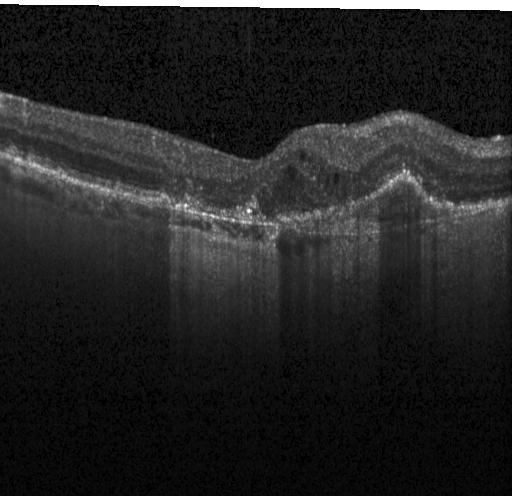 Finding: a choroidal neovascular membrane.